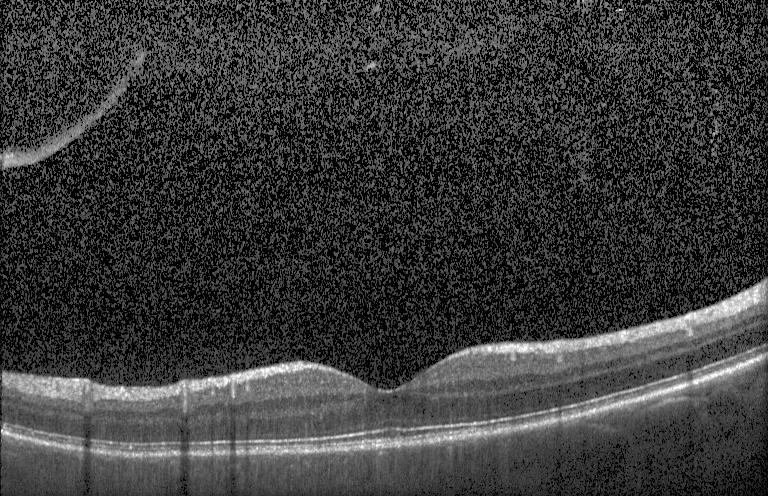 Instrument: Heidelberg Spectralis, centered on the fovea, OCT line scan. Finding: no evidence of choroidal neovascularization, diabetic macular edema, or drusen.